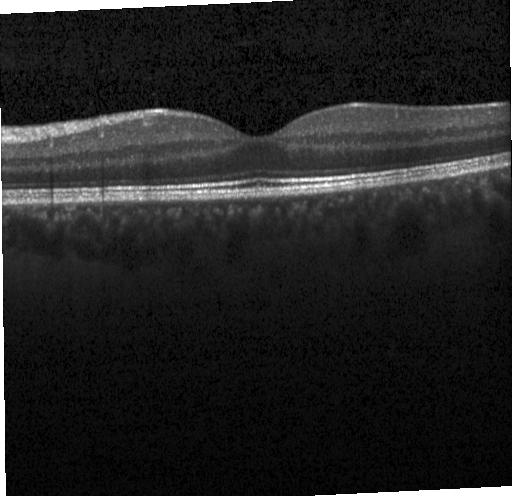

Optical coherence tomography B-scan
Neither choroidal neovascularization, diabetic macular edema, nor drusen.